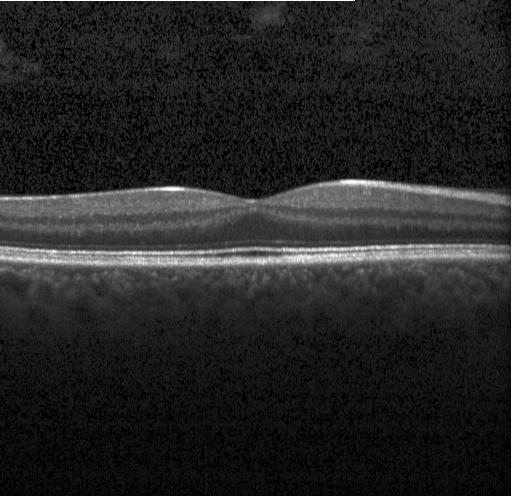

Dx: no choroidal neovascularization, no diabetic macular edema, and no drusen.